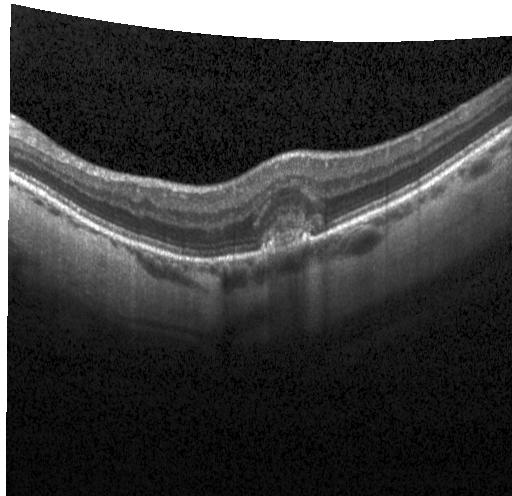 Acquired on a Heidelberg Spectralis. Optical coherence tomography scan — CNV.